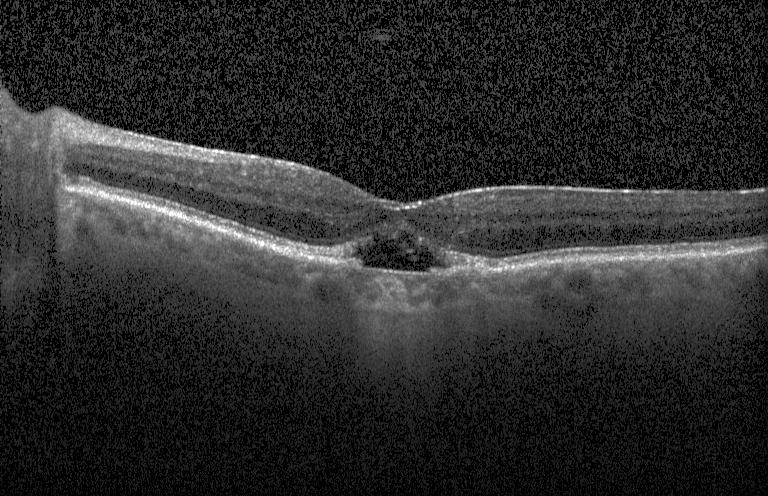

Macular OCT: CNV.